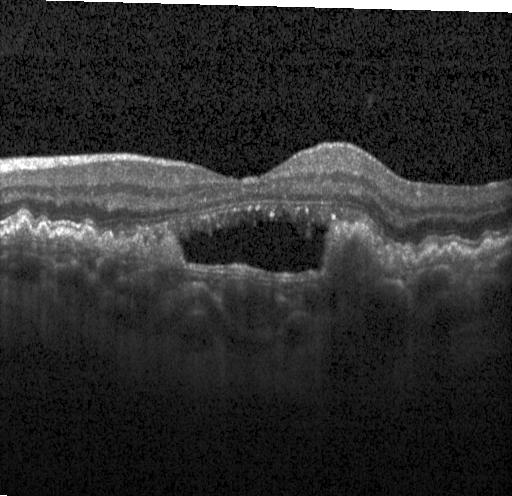

Retinal OCT cross-section · spectral-domain OCT — Dx: choroidal neovascularization (CNV).